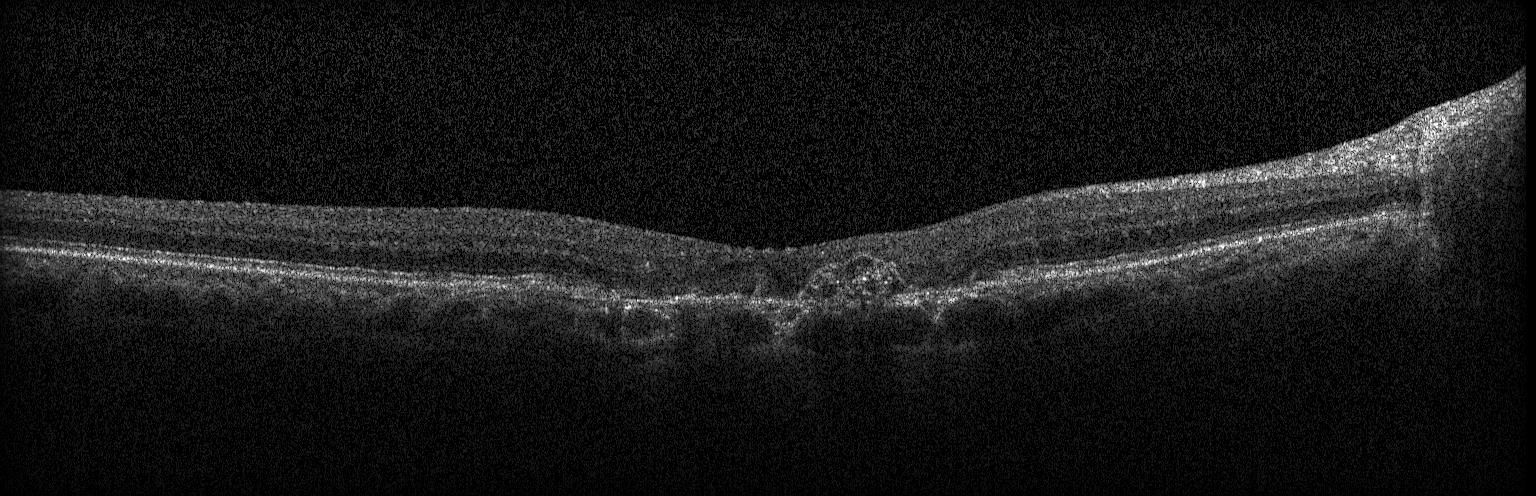
Instrument: Heidelberg Spectralis · horizontal scan through the fovea · optical coherence tomography scan · spectral-domain optical coherence tomography.
Impression: CNV.